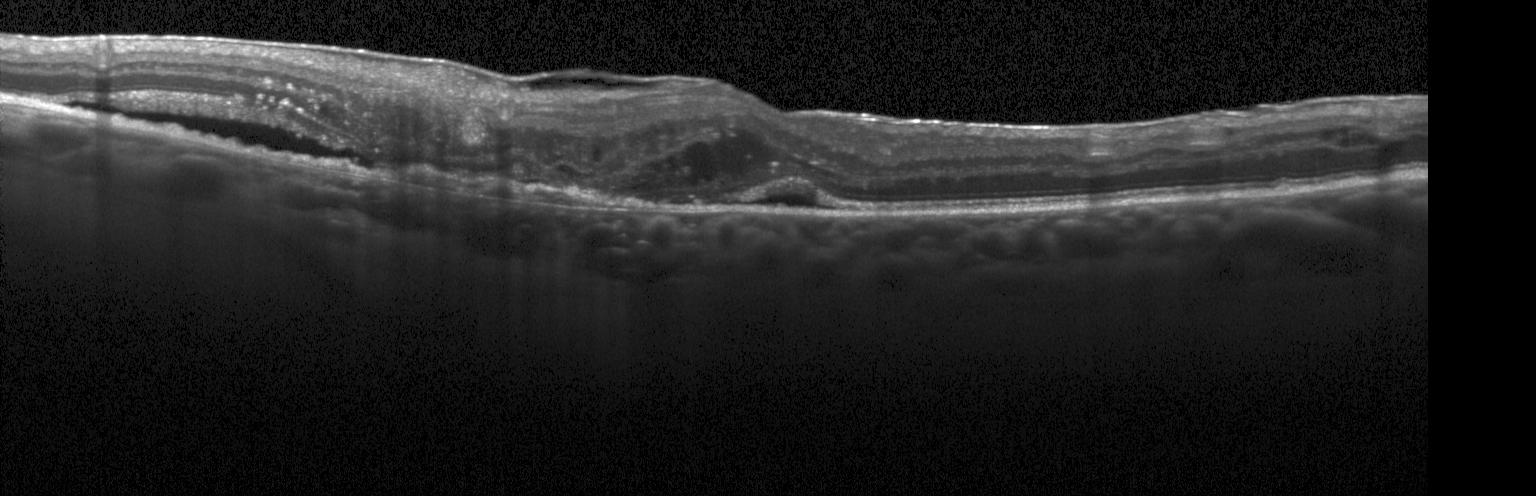
Dx: a choroidal neovascular membrane.